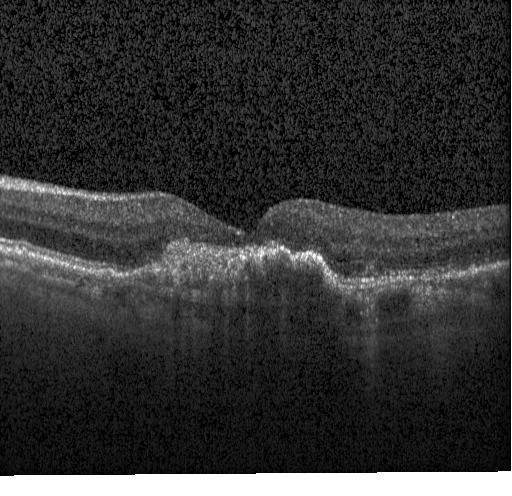 Retinal OCT B-scan
Assessment: choroidal neovascularization.